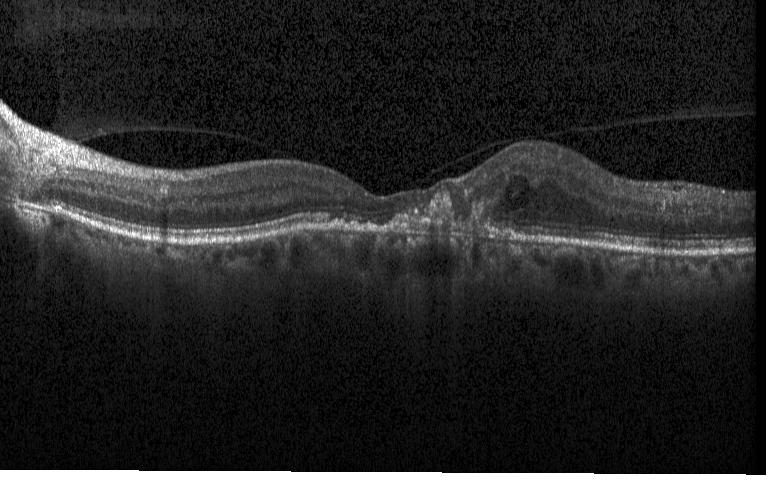
Spectral-domain optical coherence tomography · retinal OCT cross-section. The scan shows CNV.